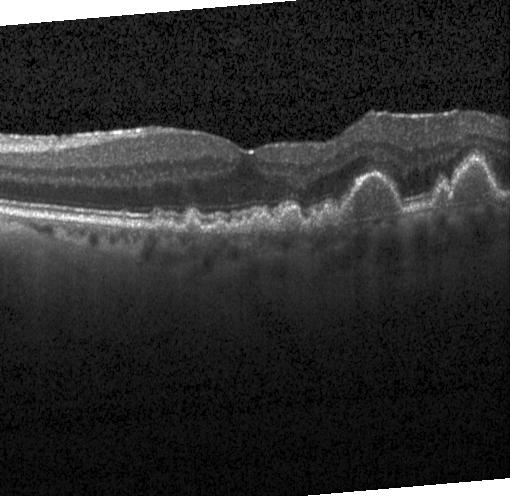

OCT line scan · macular scan · instrument: Heidelberg Spectralis
Impression: sub-RPE drusenoid deposits.